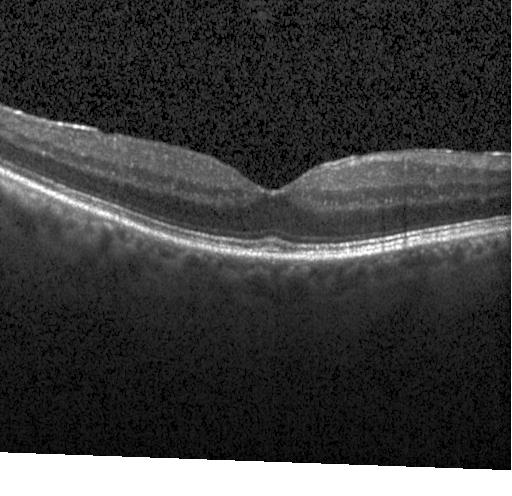
Retinal OCT B-scan — This B-scan demonstrates no evidence of choroidal neovascularization, diabetic macular edema, or drusen.